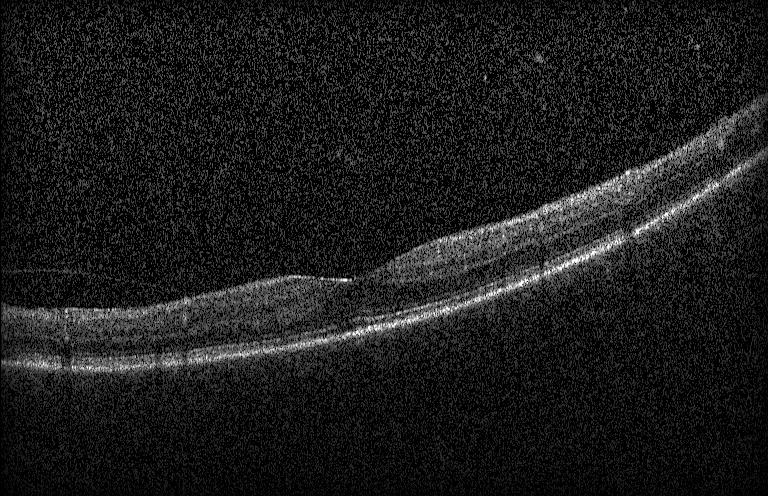

Macular OCT: no CNV, no DME, and no drusen.